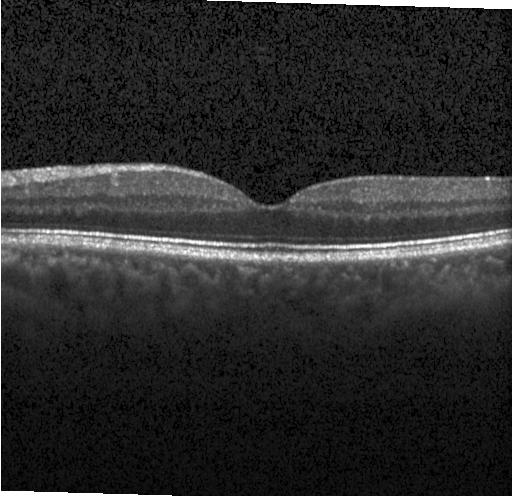 OCT line scan — Diagnosis: no choroidal neovascularization, no diabetic macular edema, and no drusen.